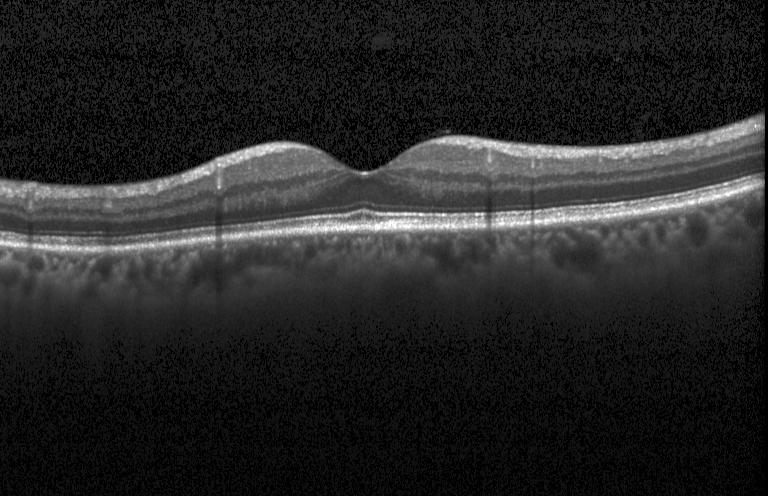
Finding: no evidence of CNV, DME, or drusen.